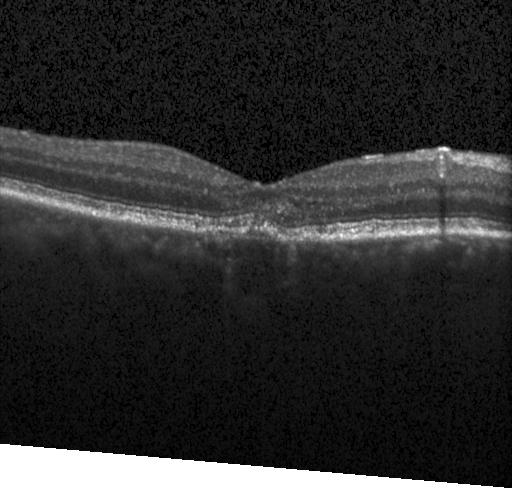 Acquired on a Heidelberg Spectralis; OCT B-scan. Impression: choroidal neovascularization.